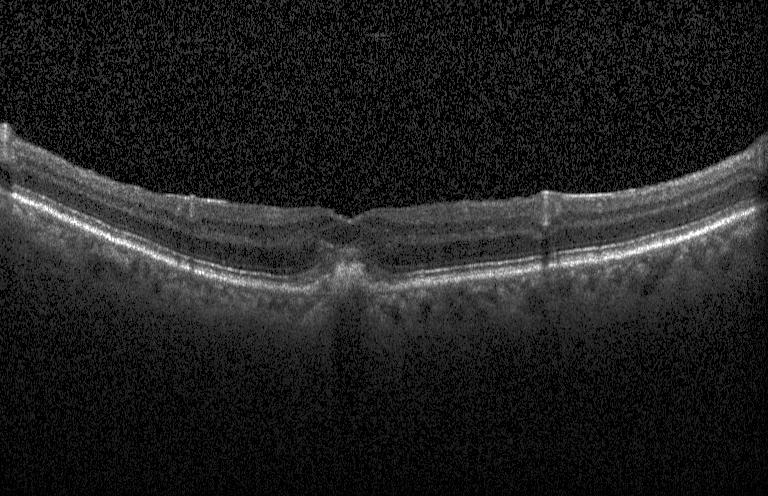

Spectral-domain OCT, optical coherence tomography B-scan. Assessment: choroidal neovascularization (CNV).